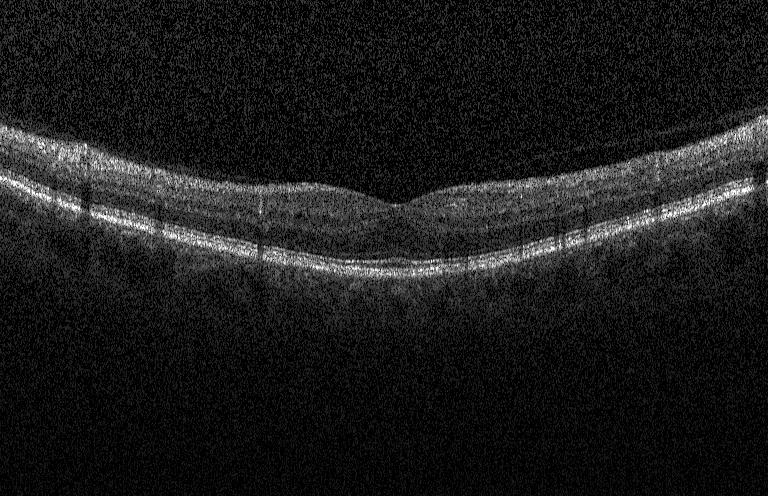 Acquired on a Heidelberg Spectralis, optical coherence tomography B-scan
OCT finding: no choroidal neovascularization, no diabetic macular edema, and no drusen.